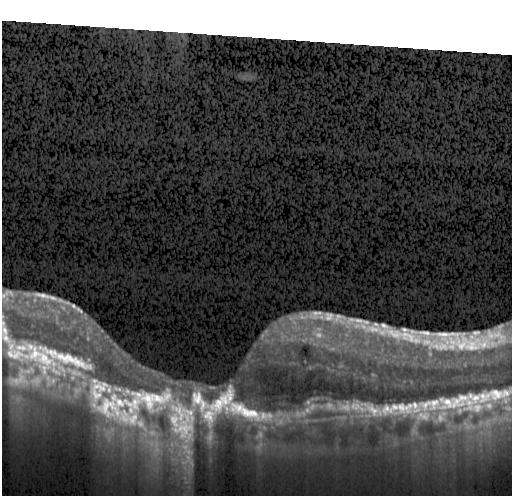 Retinal OCT cross-section. SD-OCT. Heidelberg Spectralis OCT system.
Dx: a choroidal neovascular membrane.